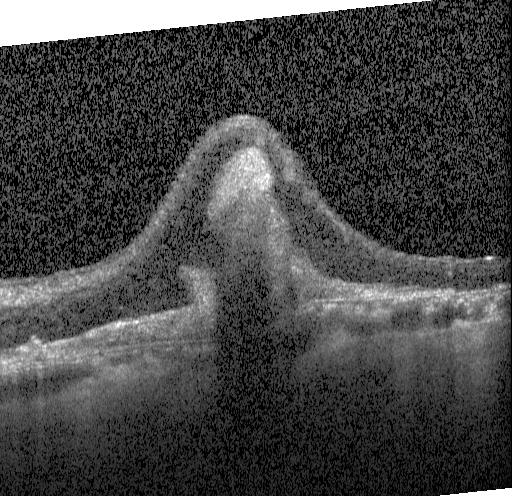 Spectral-domain optical coherence tomography · optical coherence tomography B-scan
Diagnosis: CNV.